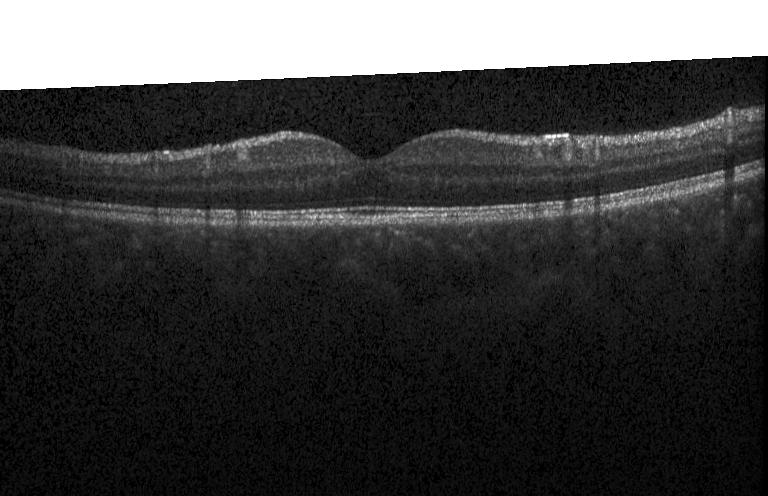 Retinal OCT B-scan; macular scan
The scan shows neither choroidal neovascularization, diabetic macular edema, nor drusen.